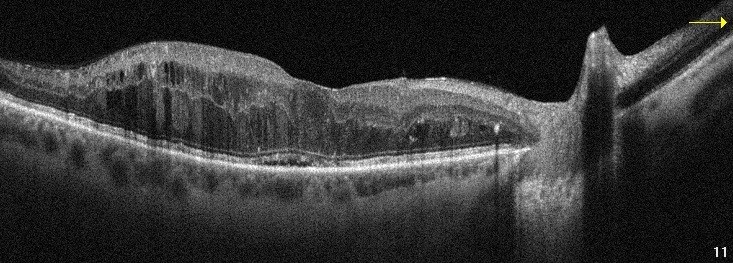
Retinal OCT cross-section; instrument: Optovue Avanti RTVue XR.
Impression: DME.